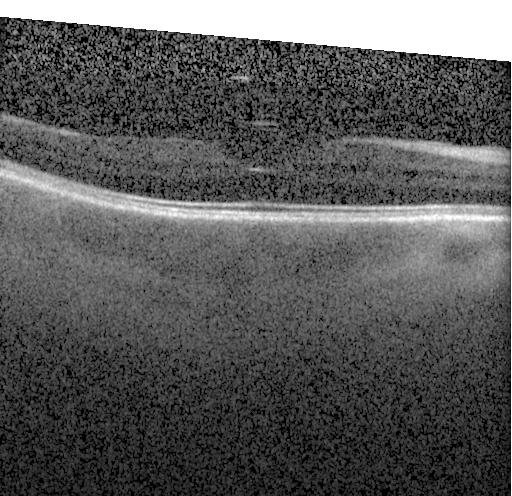

Dx: no choroidal neovascularization, diabetic macular edema, or drusen.